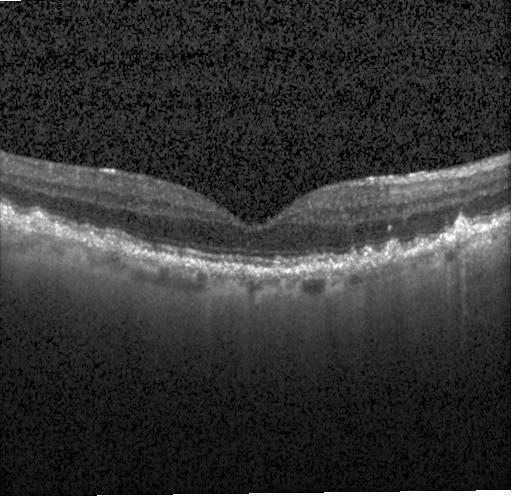 Retinal OCT cross-section · Heidelberg Spectralis OCT system. Diagnosis: sub-RPE drusenoid deposits.